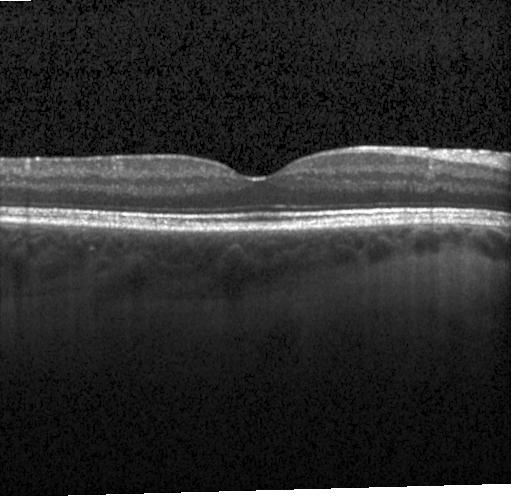 OCT line scan. Instrument: Heidelberg Spectralis. Through the macula. Spectral-domain OCT
Assessment: no choroidal neovascularization, no diabetic macular edema, and no drusen.